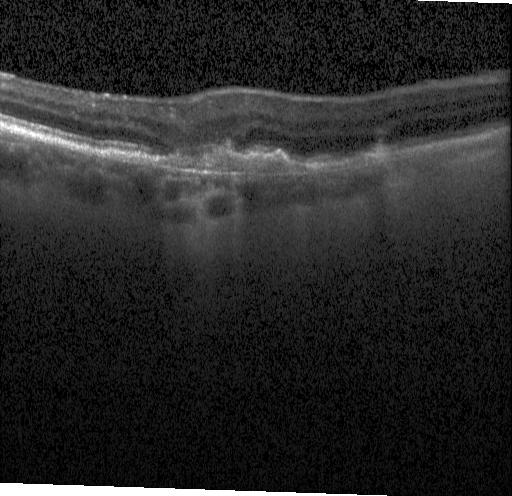 OCT line scan
A choroidal neovascular membrane.